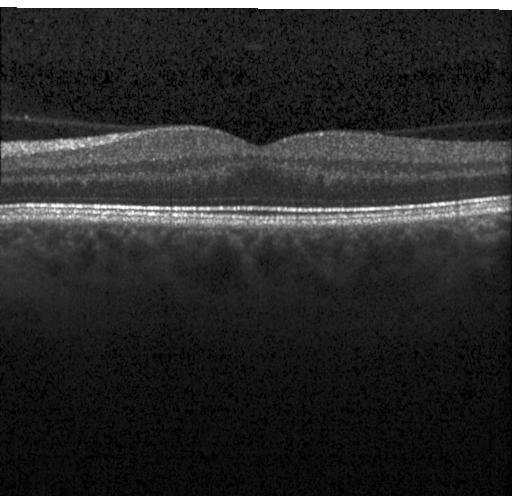
No choroidal neovascularization, no diabetic macular edema, and no drusen.